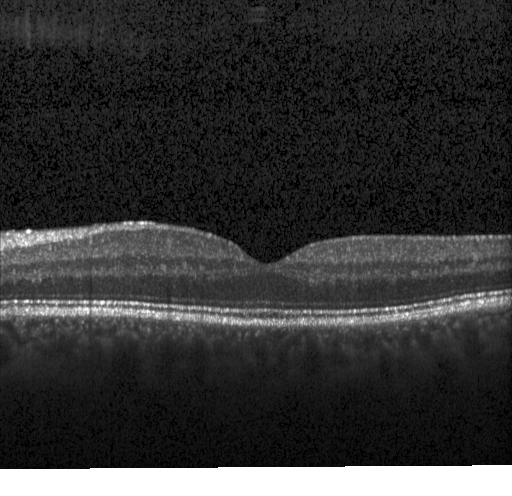

Diagnosis: no CNV, DME, or drusen.